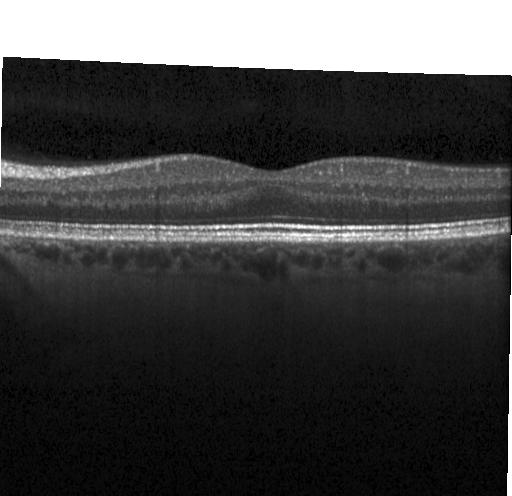

Through the macula · SD-OCT · Heidelberg Spectralis · optical coherence tomography scan.
Assessment: no choroidal neovascularization, no diabetic macular edema, and no drusen.